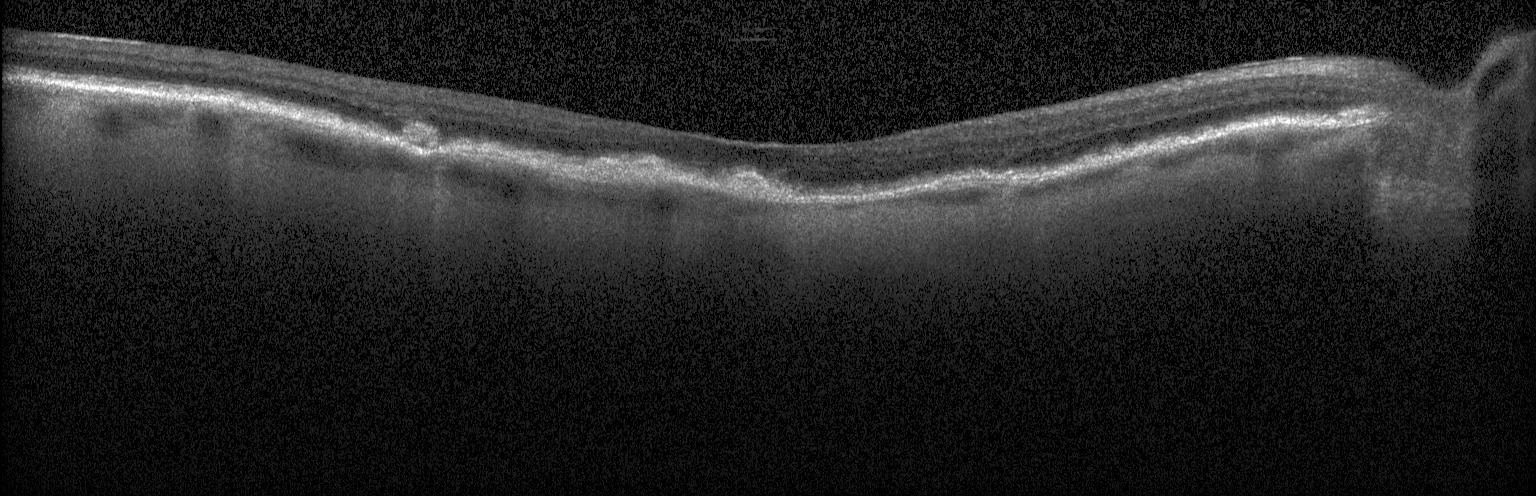 Heidelberg Spectralis. Through the macula. Retinal OCT cross-section. Macular OCT: choroidal neovascularization (CNV).